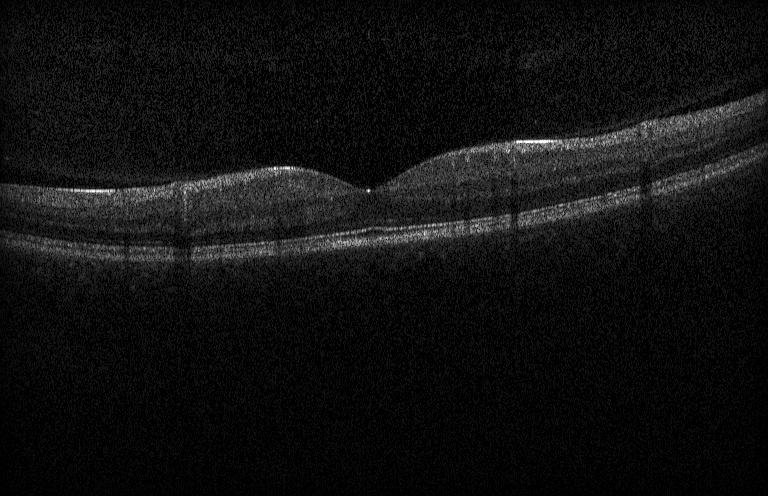
This B-scan demonstrates no evidence of CNV, DME, or drusen.